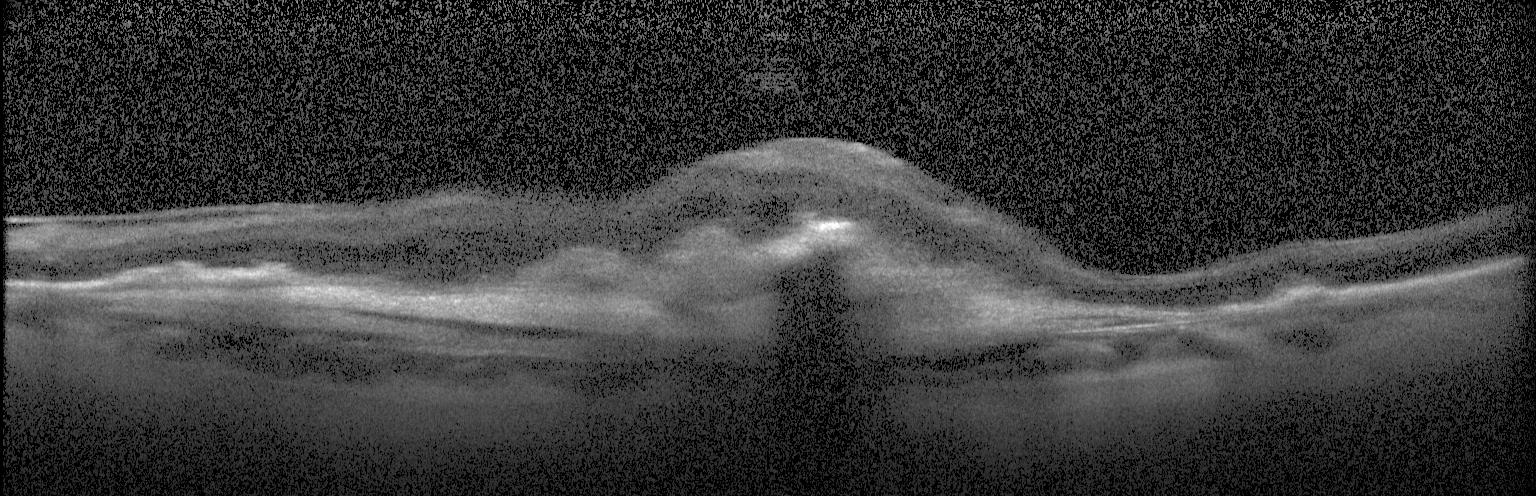

OCT B-scan.
The scan shows choroidal neovascularization (CNV).